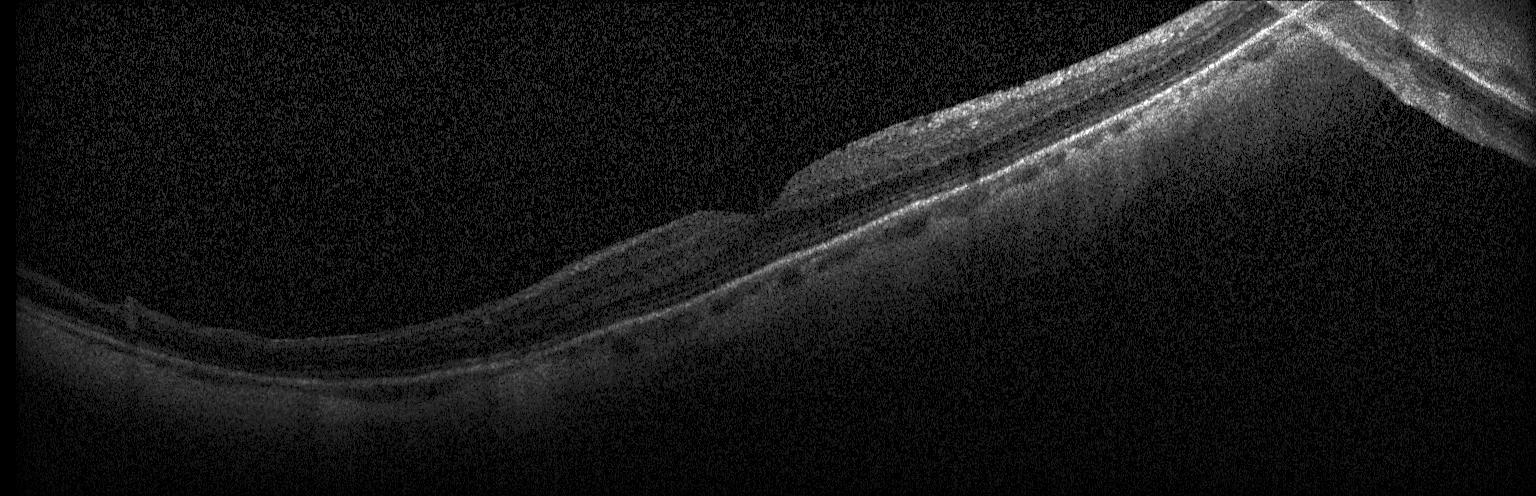

Retinal OCT cross-section. Diagnosis: no choroidal neovascularization, no diabetic macular edema, and no drusen.